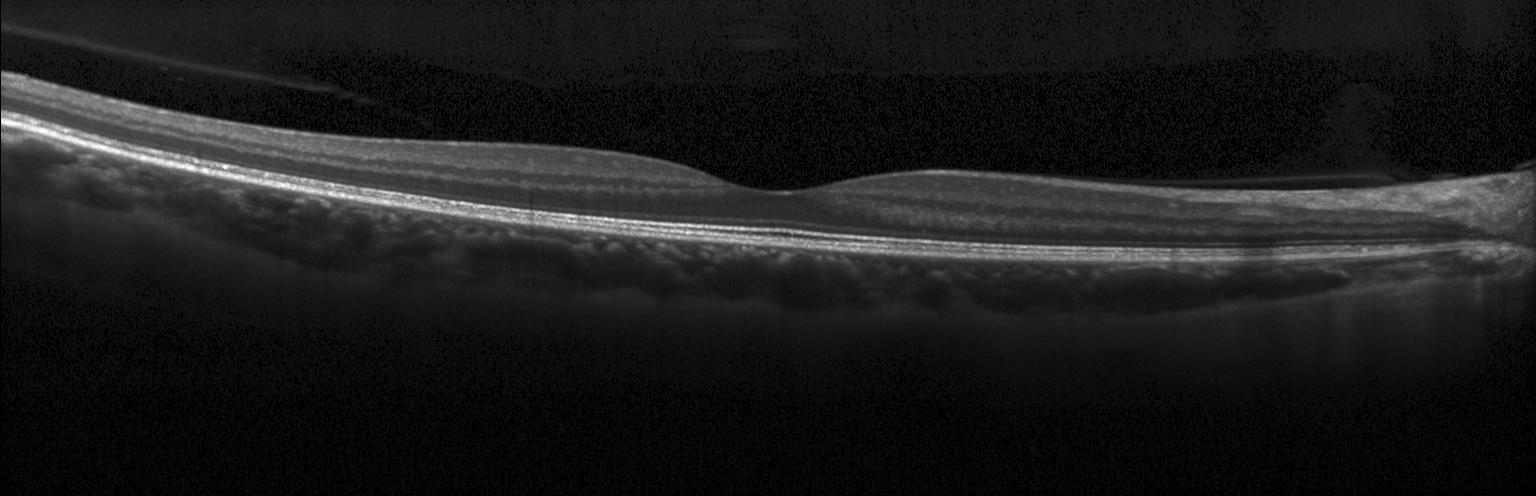 Retinal OCT cross-section. Neither choroidal neovascularization, diabetic macular edema, nor drusen.